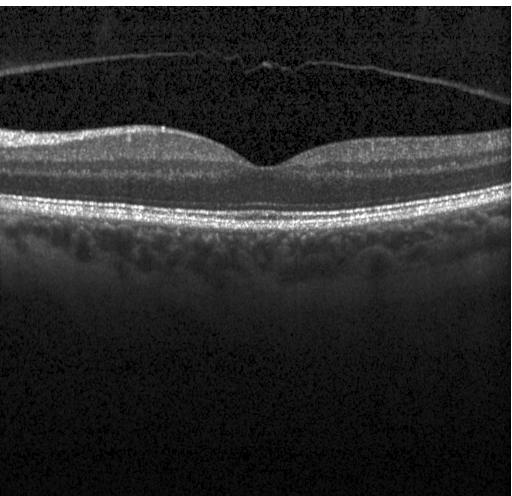

Finding: no choroidal neovascularization, diabetic macular edema, or drusen.